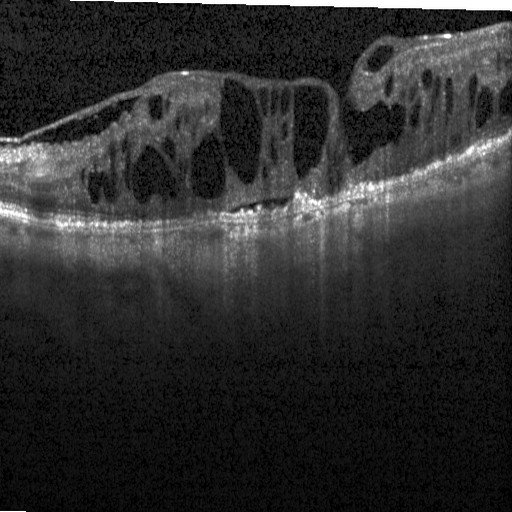
Retinal OCT cross-section, Heidelberg Spectralis OCT system. DME.